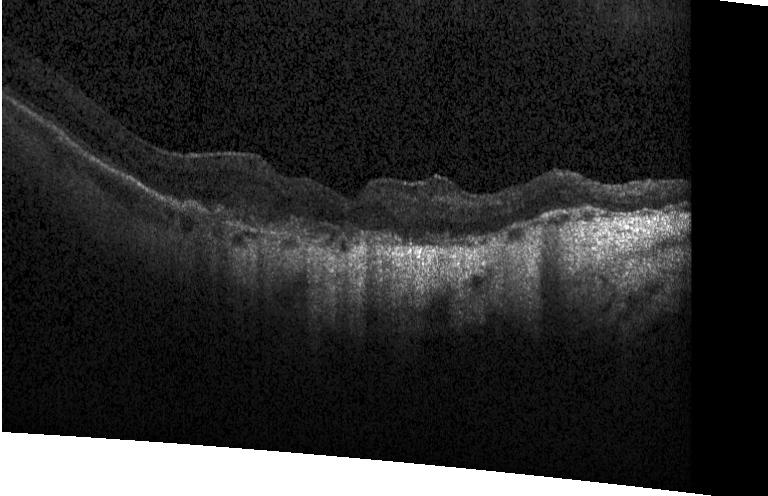

Retinal OCT cross-section showing CNV.